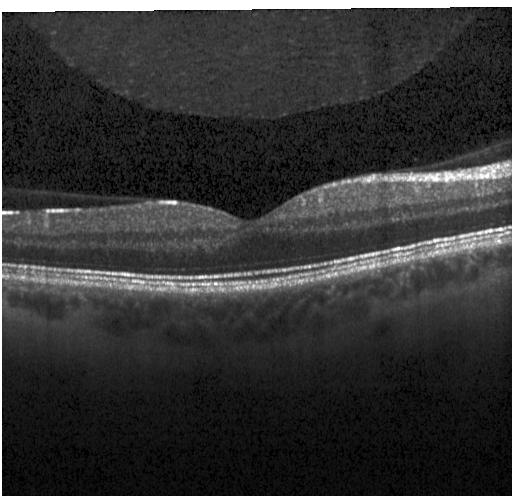
Diagnosis: neither choroidal neovascularization, diabetic macular edema, nor drusen.